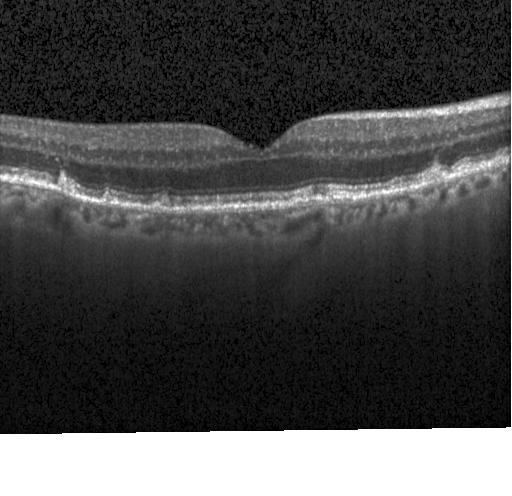

Impression: sub-RPE drusenoid deposits.